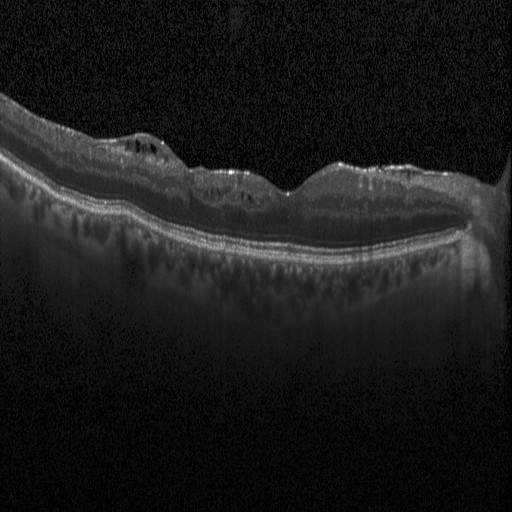

Retinal OCT cross-section
Dx: DME.